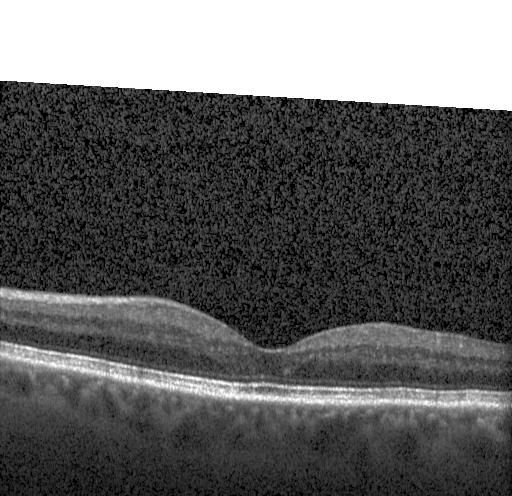 Through the macula · SD-OCT · optical coherence tomography B-scan · acquired on a Heidelberg Spectralis
Impression: neither choroidal neovascularization, diabetic macular edema, nor drusen.